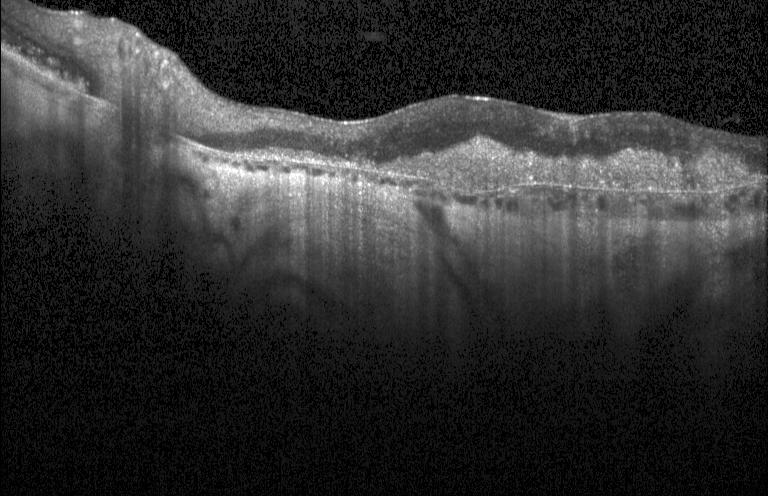 OCT B-scan showing a choroidal neovascular membrane.